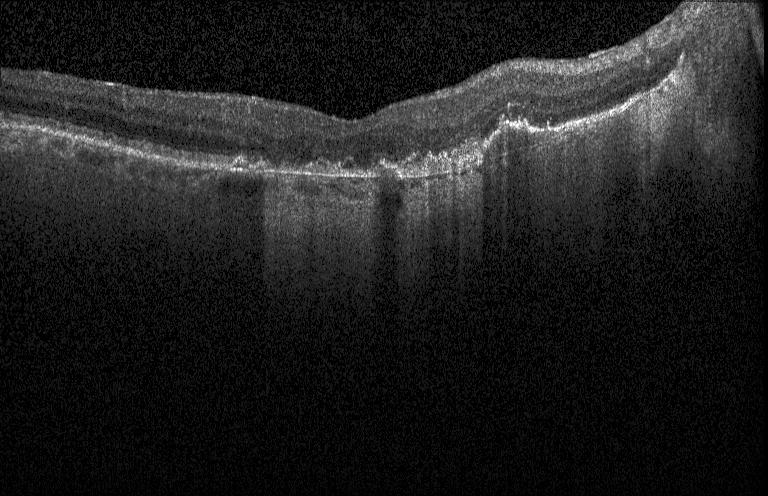 This B-scan demonstrates CNV.